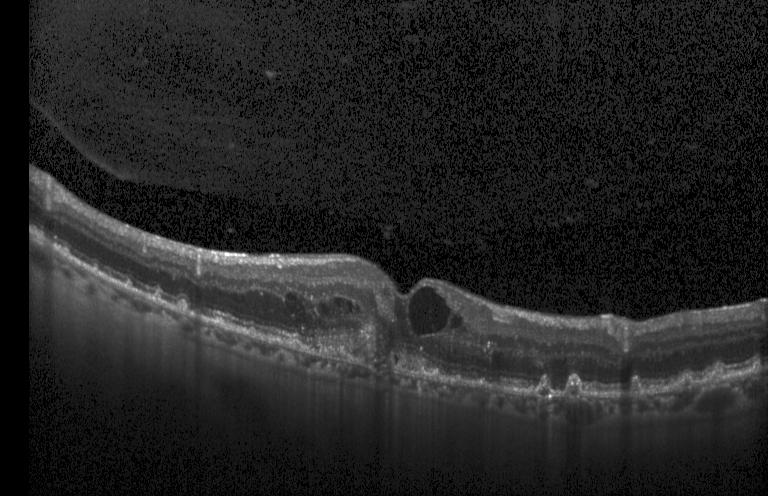 Diagnosis: choroidal neovascularization (CNV).